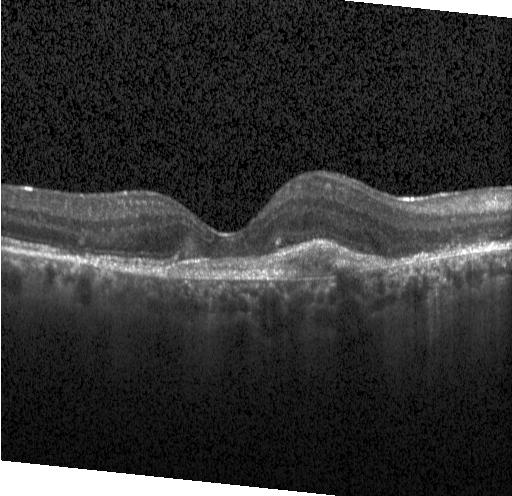
Optical coherence tomography B-scan — The scan shows a choroidal neovascular membrane.